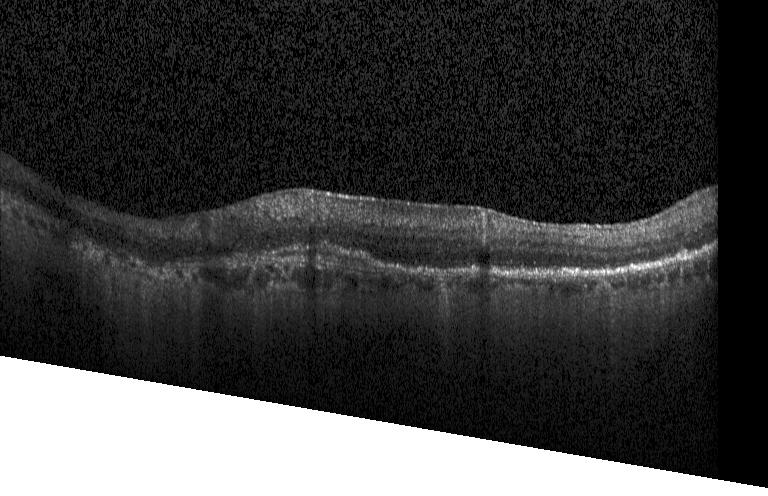
The scan shows a choroidal neovascular membrane.